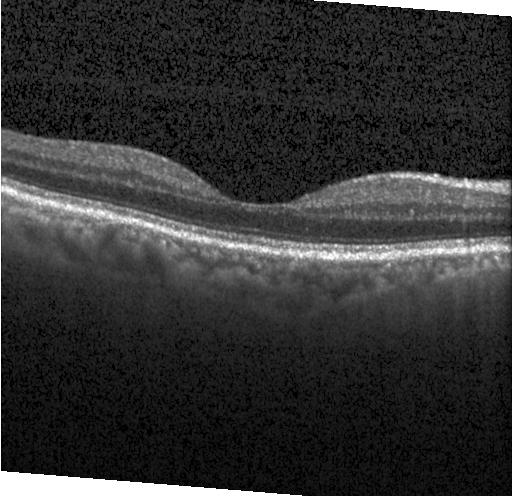
Diagnosis: no evidence of choroidal neovascularization, diabetic macular edema, or drusen.